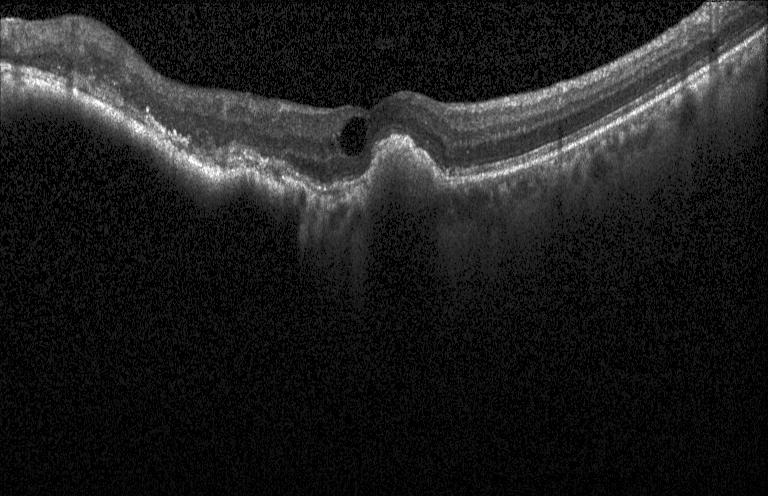
Instrument: Heidelberg Spectralis. SD-OCT. OCT B-scan. Centered on the fovea — Assessment: choroidal neovascularization.